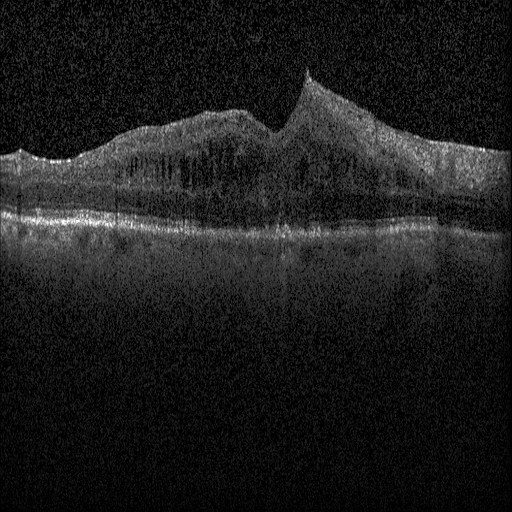 OCT B-scan
Finding: diabetic macular edema.